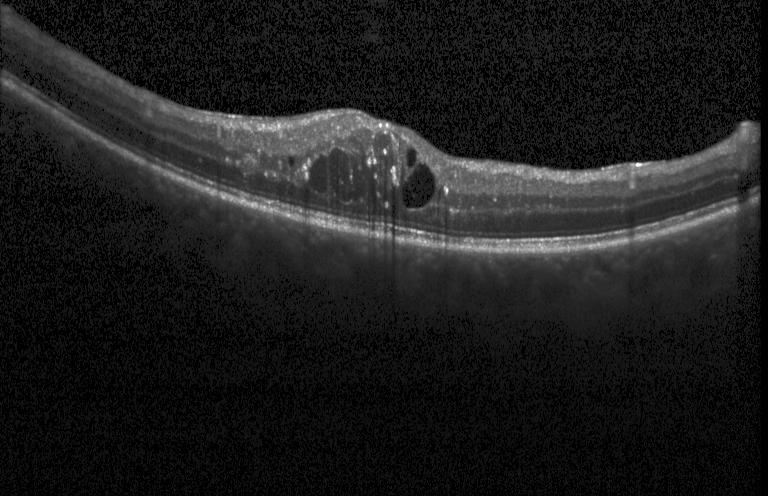

This B-scan demonstrates diabetic macular edema.